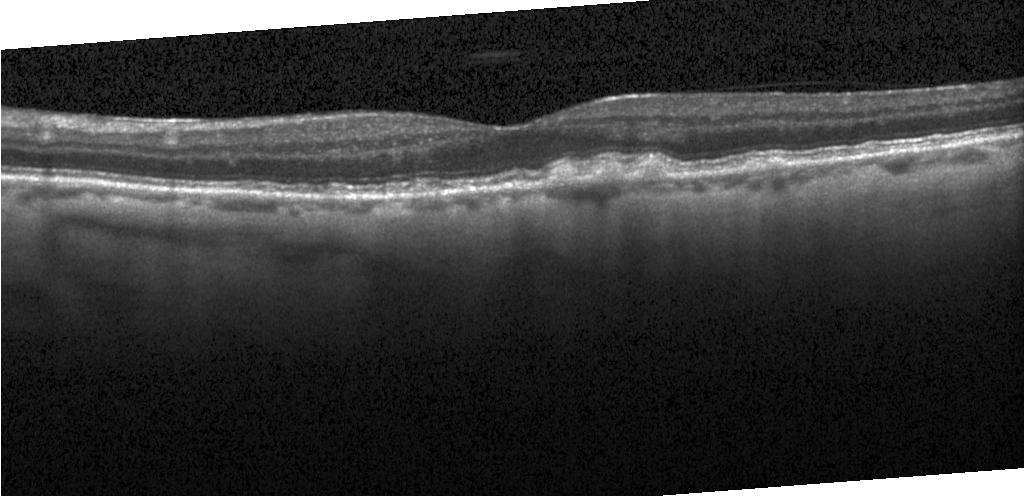
Fovea-centered, spectral-domain OCT, OCT line scan. Impression: multiple drusen.